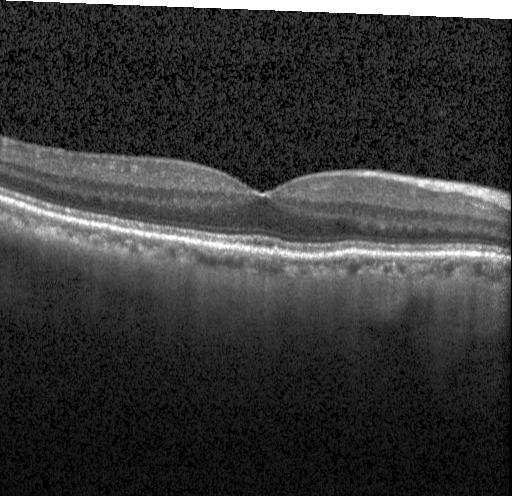

OCT line scan. Spectral-domain optical coherence tomography.
Finding: no evidence of choroidal neovascularization, diabetic macular edema, or drusen.